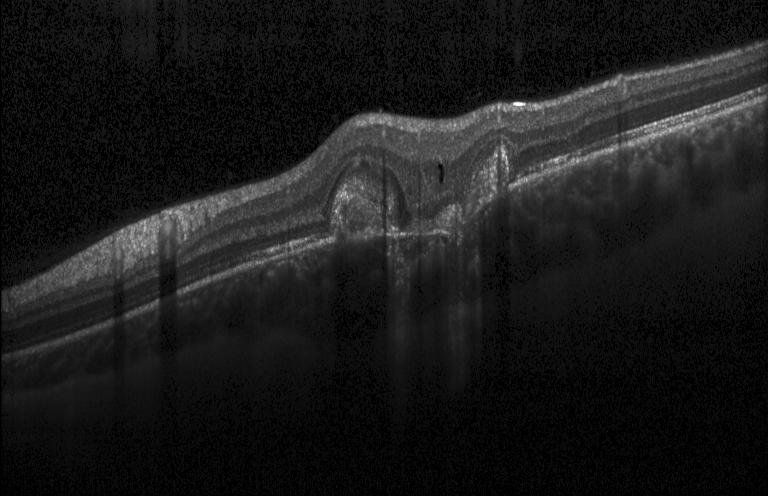

OCT B-scan. Spectral-domain OCT — Diagnosis: a choroidal neovascular membrane.